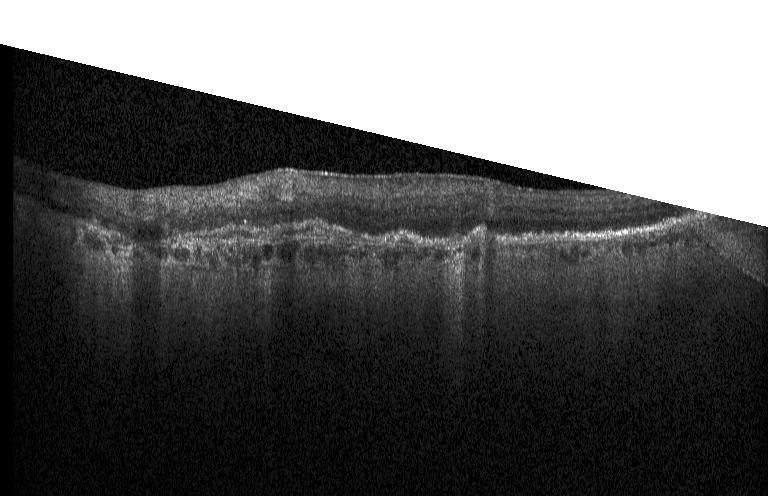
OCT B-scan showing a choroidal neovascular membrane.